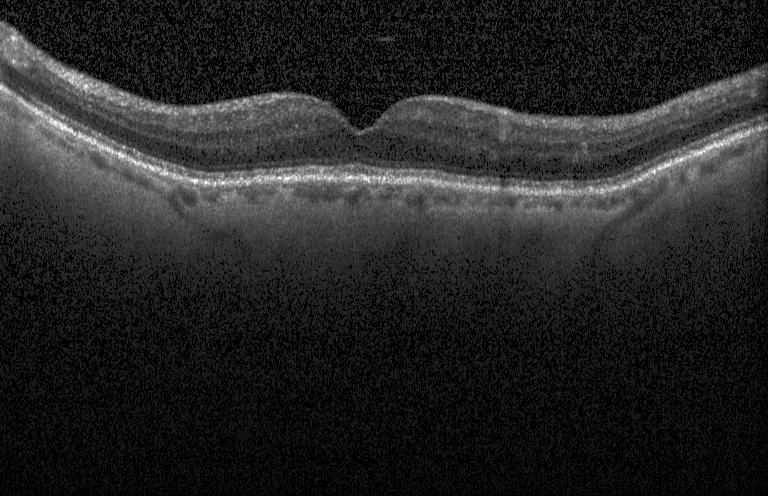 Retinal OCT cross-section; Heidelberg Spectralis; through the macula — This B-scan demonstrates neither choroidal neovascularization, diabetic macular edema, nor drusen.